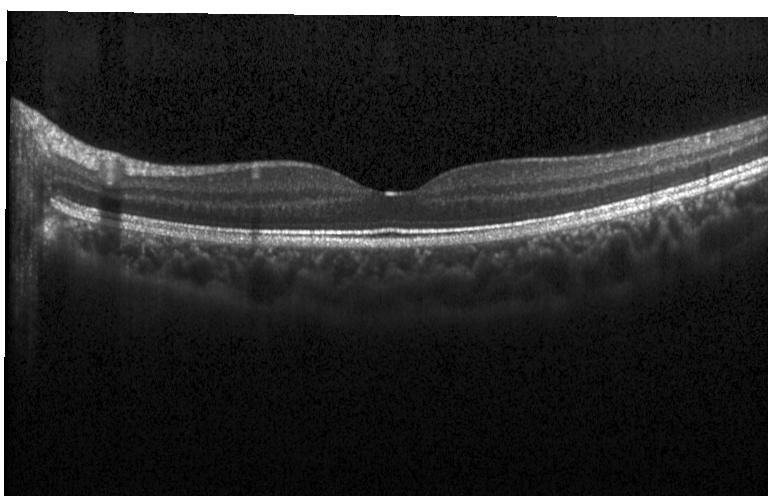

OCT finding: no evidence of CNV, DME, or drusen.